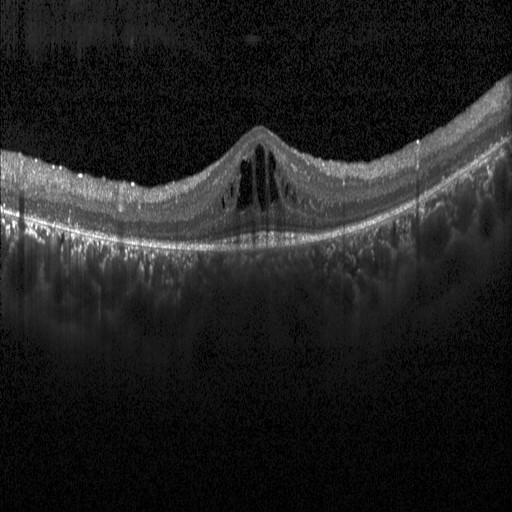

Finding: diabetic macular edema (DME).